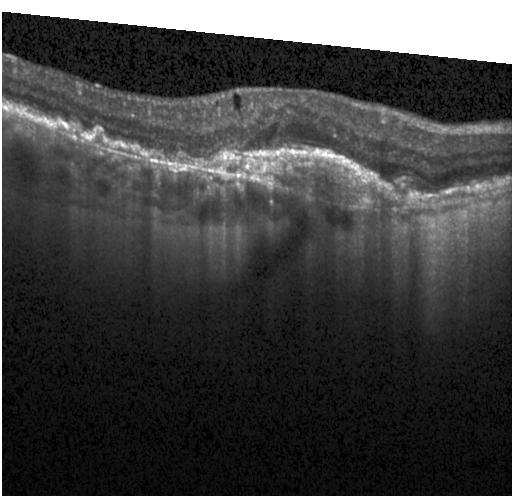

Optical coherence tomography B-scan. Impression: a choroidal neovascular membrane.